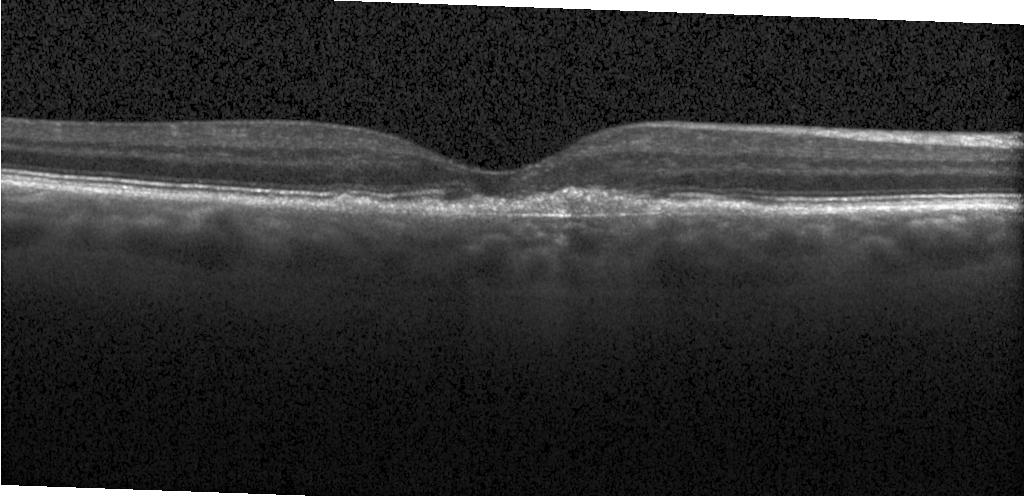
Retinal OCT cross-section — The scan shows CNV.